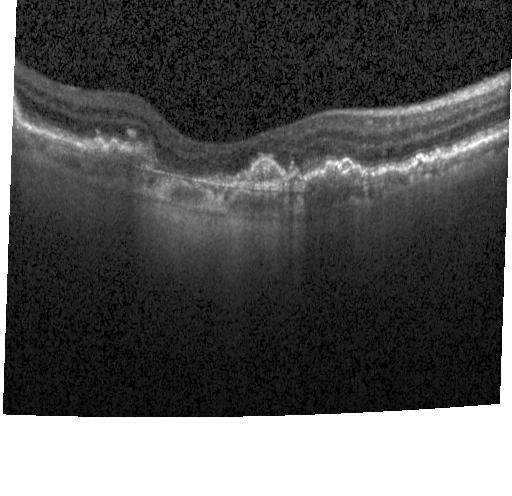 Macular OCT demonstrating a choroidal neovascular membrane.